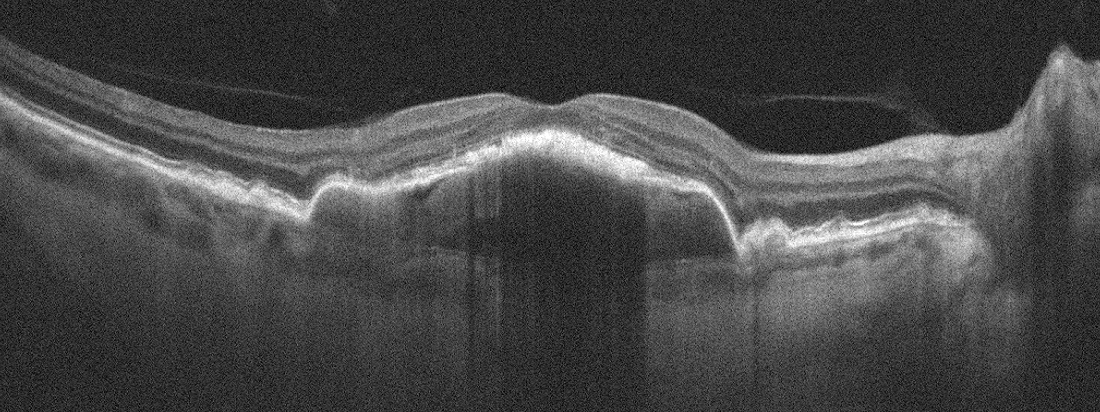 Optovue Avanti RTVue XR · retinal OCT cross-section · macular scan. Impression: age-related macular degeneration (AMD).